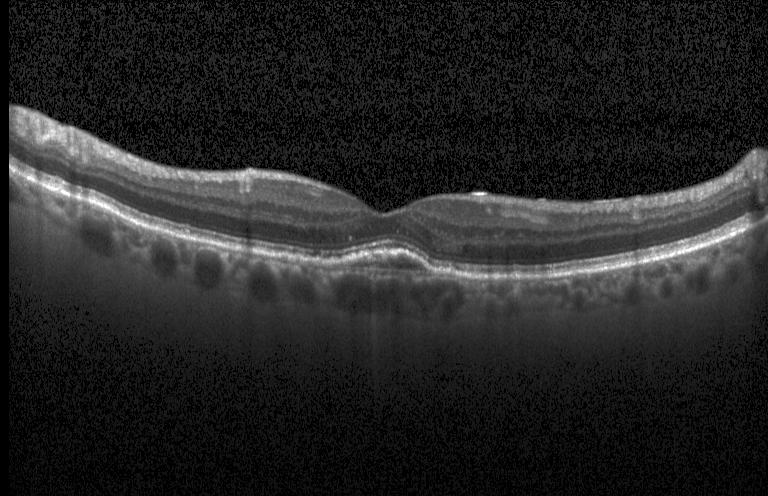 Assessment: a choroidal neovascular membrane.